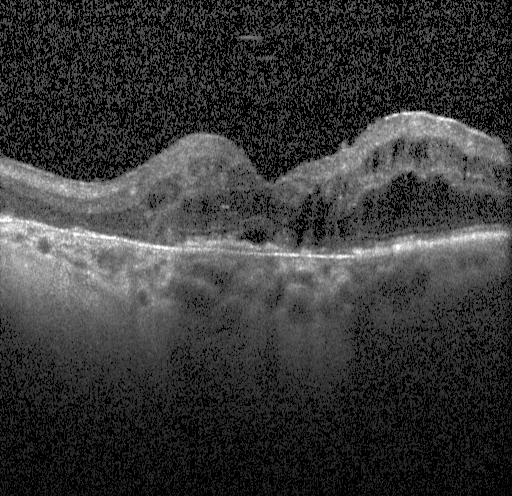
Fovea-centered. Optical coherence tomography B-scan. Spectral-domain OCT — Diagnosis: a choroidal neovascular membrane.